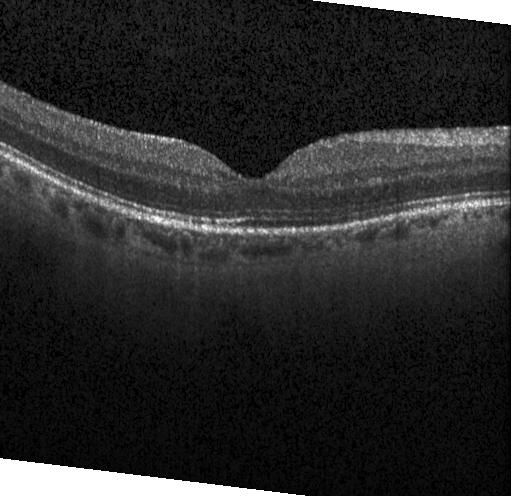

Macular OCT demonstrating no choroidal neovascularization, no diabetic macular edema, and no drusen.